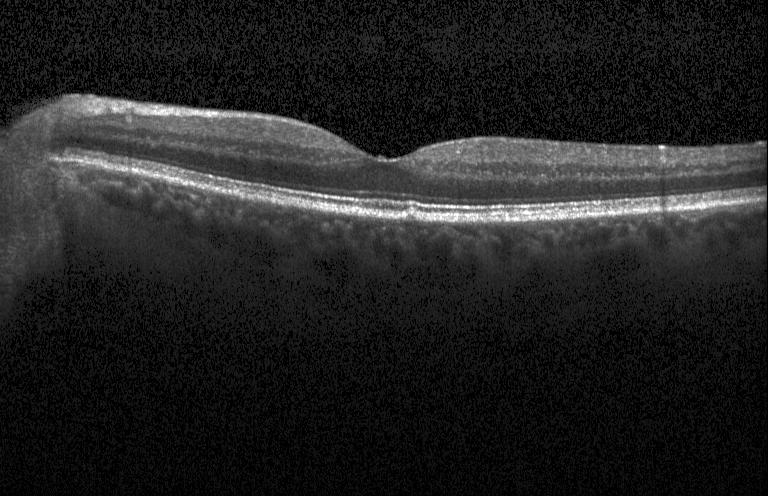 Heidelberg Spectralis · OCT line scan · SD-OCT. Diagnosis: sub-RPE drusenoid deposits.